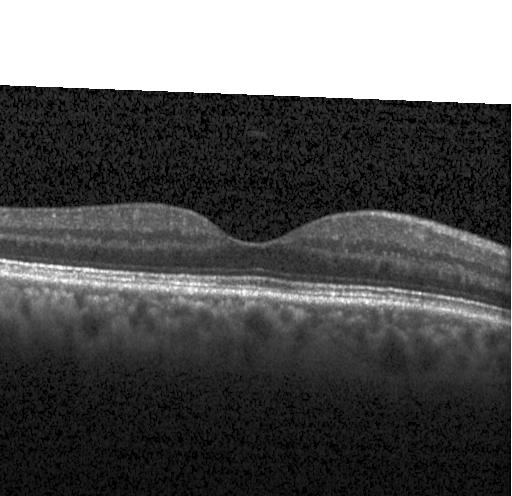 Spectral-domain OCT B-scan: neither CNV, DME, nor drusen.